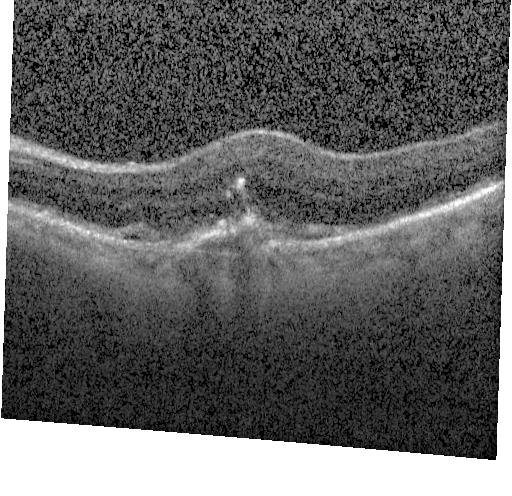
A choroidal neovascular membrane.